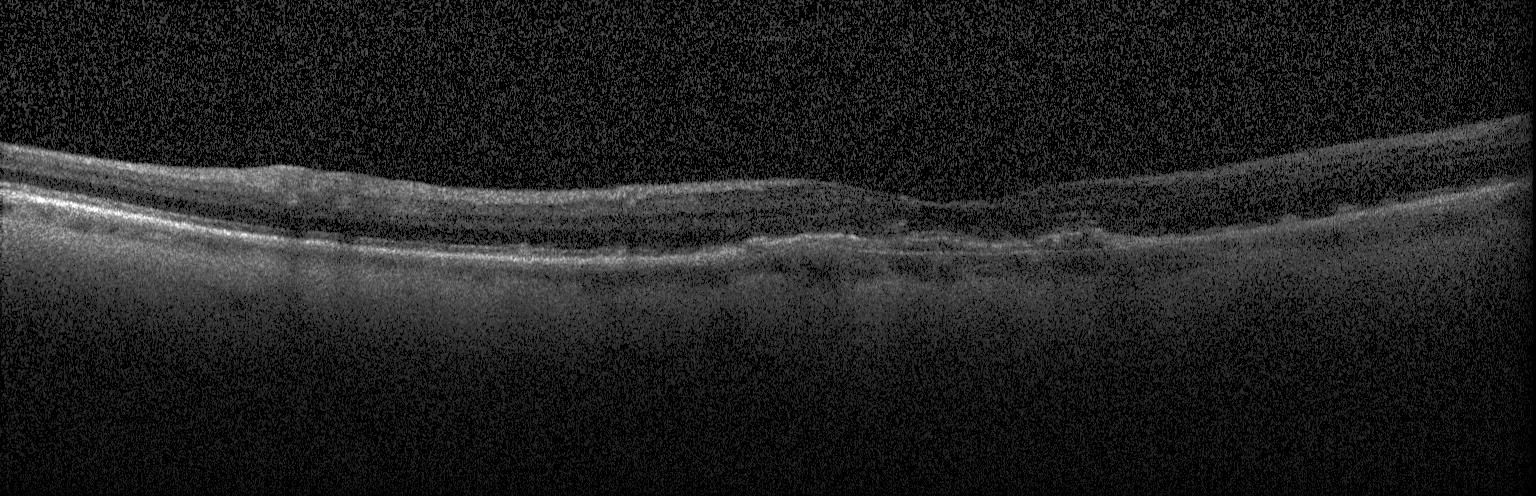

Retinal OCT B-scan · SD-OCT
Finding: a choroidal neovascular membrane.